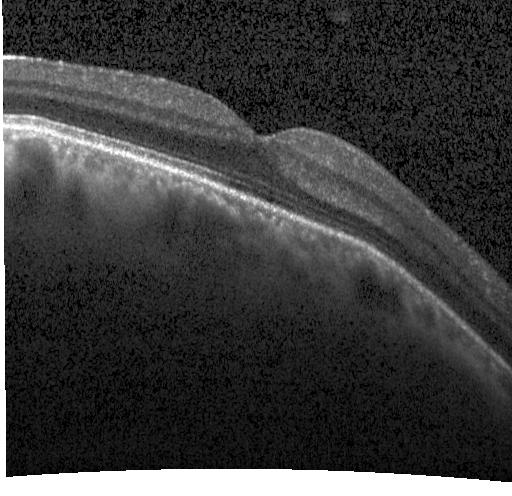

Diagnosis: neither choroidal neovascularization, diabetic macular edema, nor drusen.